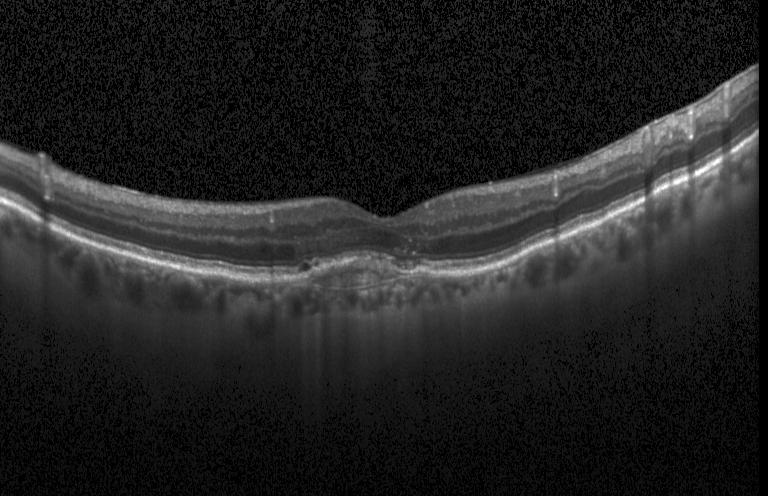

OCT B-scan.
Impression: choroidal neovascularization.